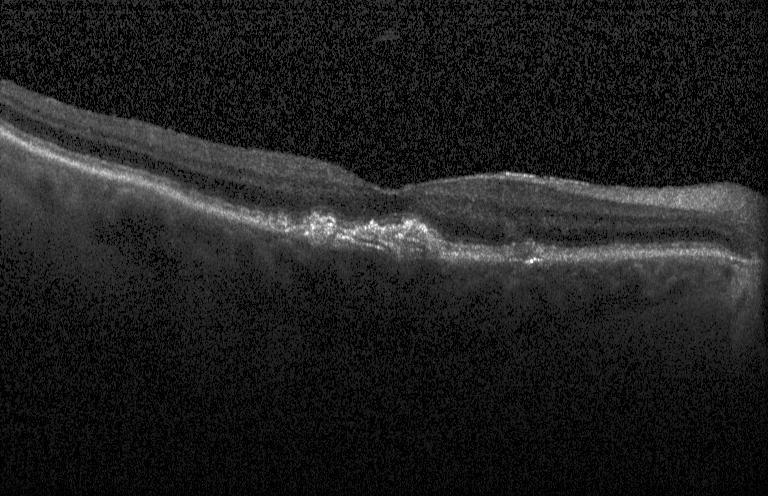

Macular scan; retinal OCT cross-section
OCT finding: CNV.